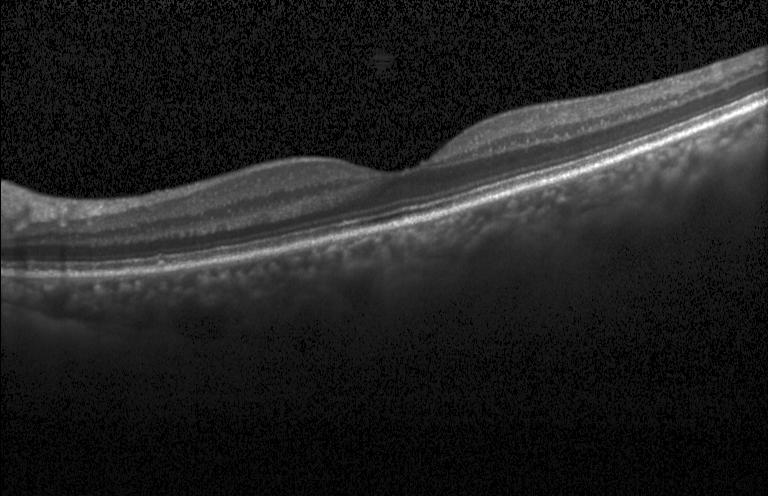
Instrument: Heidelberg Spectralis · OCT line scan · SD-OCT
Impression: no evidence of choroidal neovascularization, diabetic macular edema, or drusen.